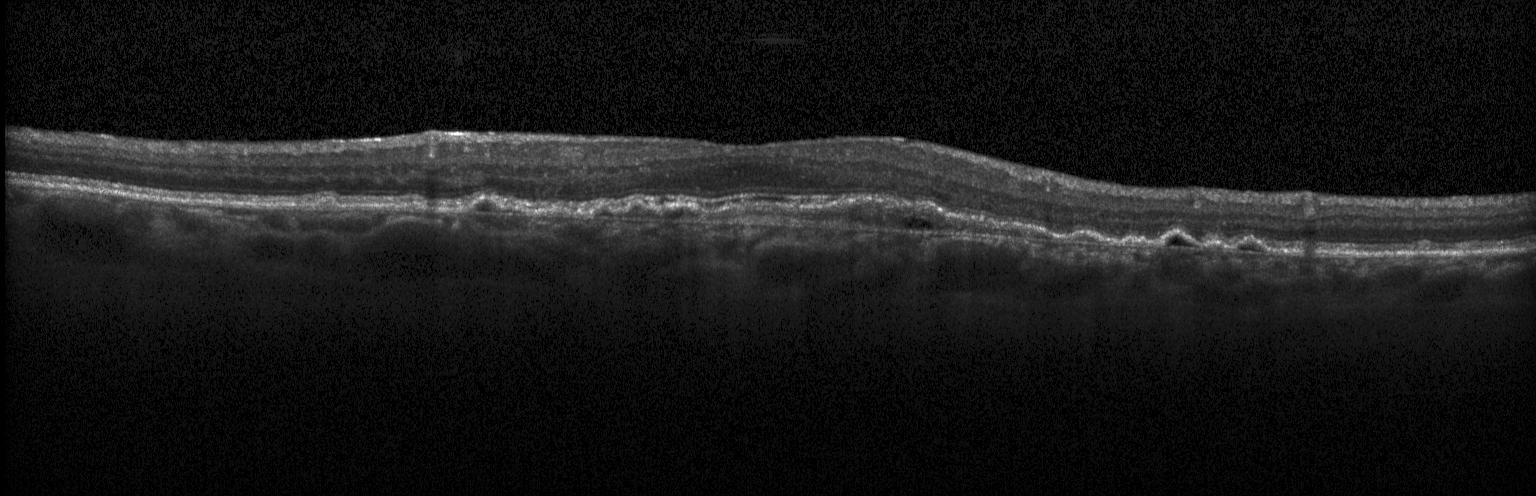 Retinal OCT B-scan. Diagnosis: choroidal neovascularization.